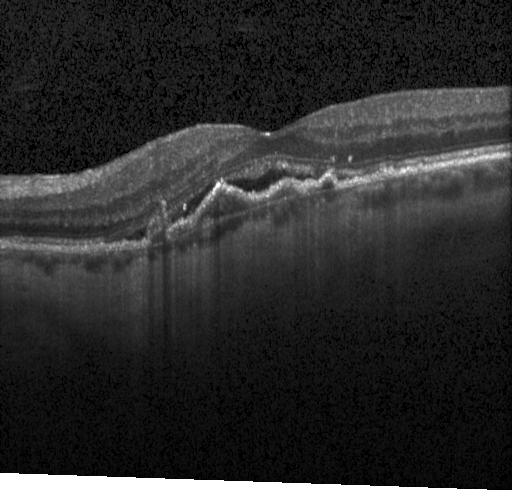
Finding: a choroidal neovascular membrane.